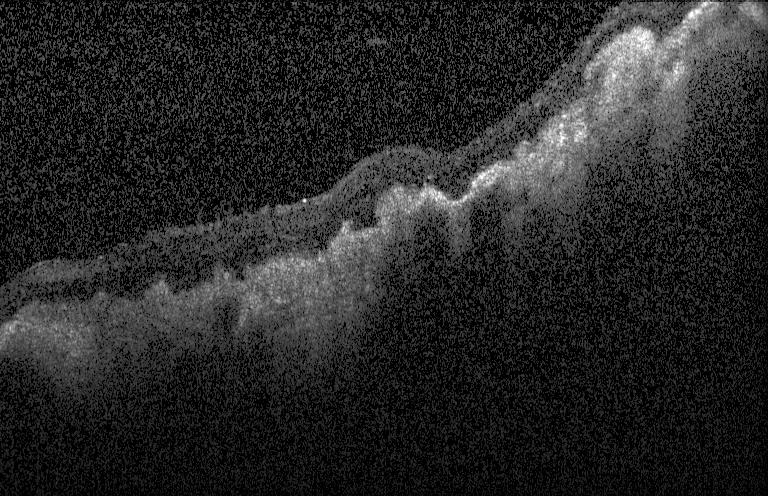
The scan shows a choroidal neovascular membrane.